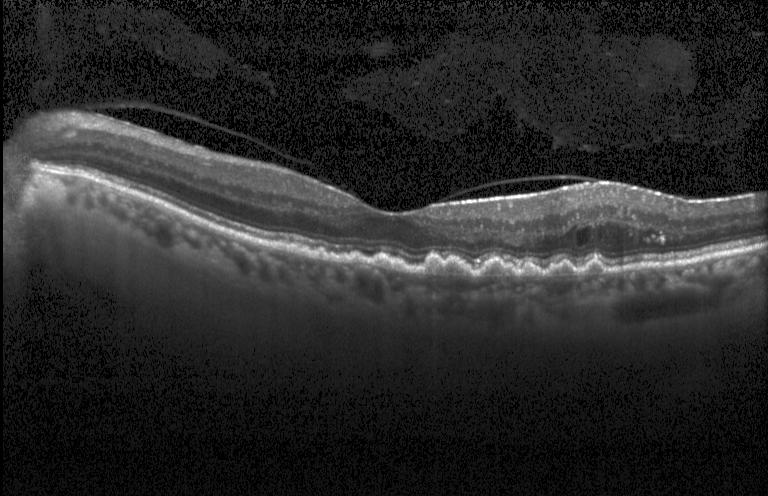
This B-scan demonstrates choroidal neovascularization (CNV).